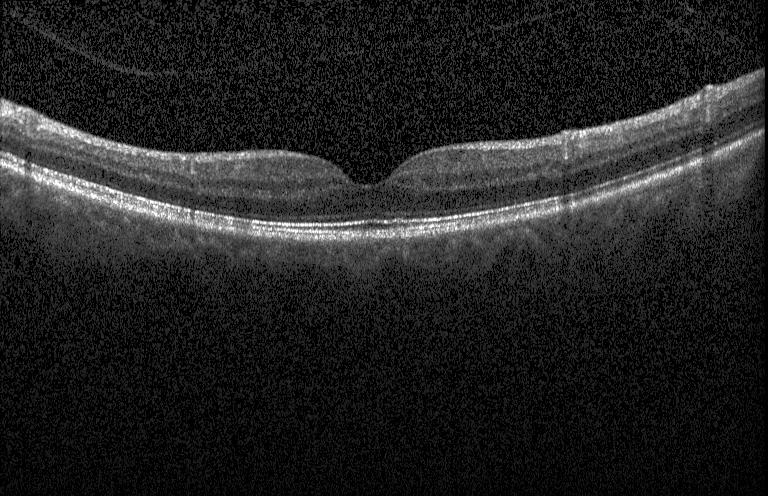
OCT line scan; fovea-centered
This B-scan demonstrates neither CNV, DME, nor drusen.